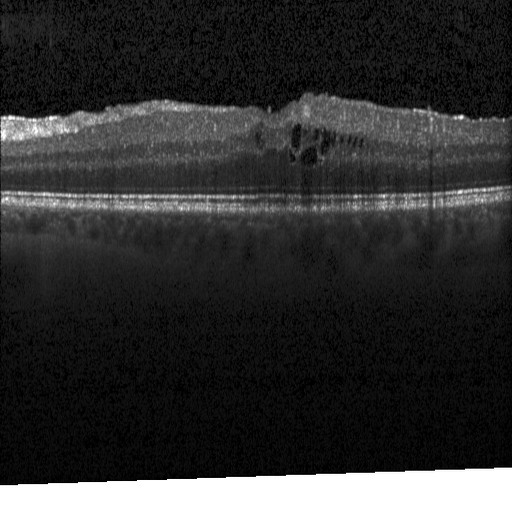 Retinal OCT cross-section — Impression: diabetic macular edema (DME).